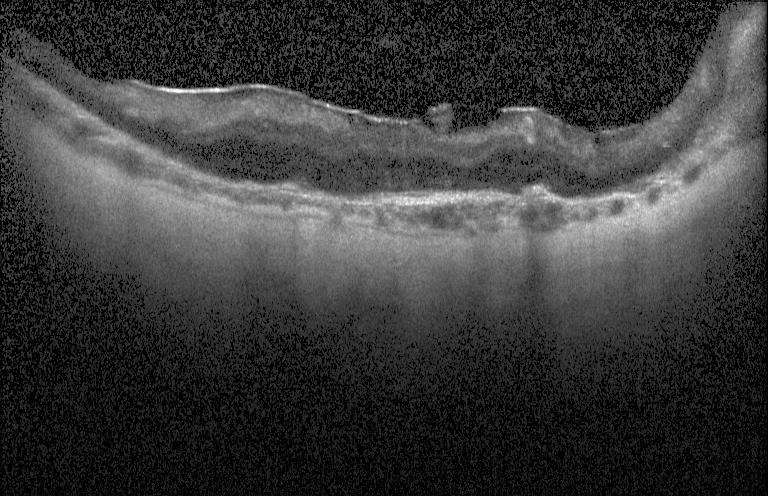
Diagnosis: a choroidal neovascular membrane.